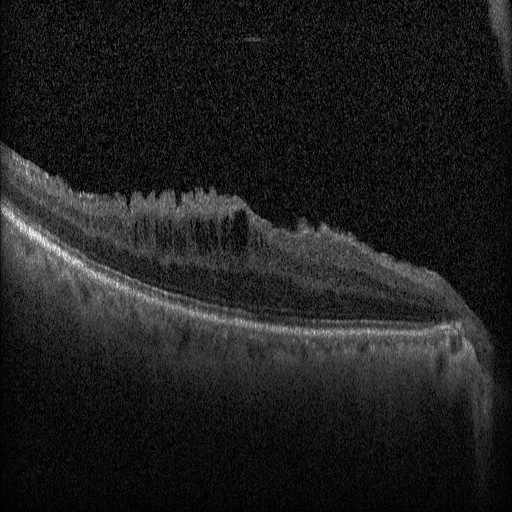

Heidelberg Spectralis OCT system; optical coherence tomography B-scan; SD-OCT — Finding: diabetic macular edema.